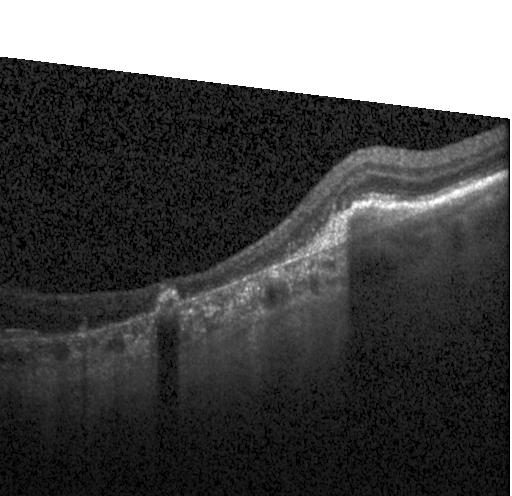 Impression: CNV.